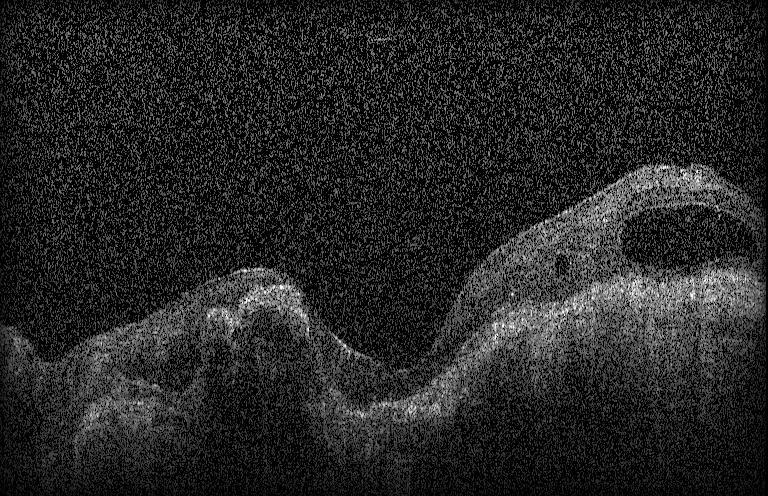

Heidelberg Spectralis, OCT B-scan.
A choroidal neovascular membrane.